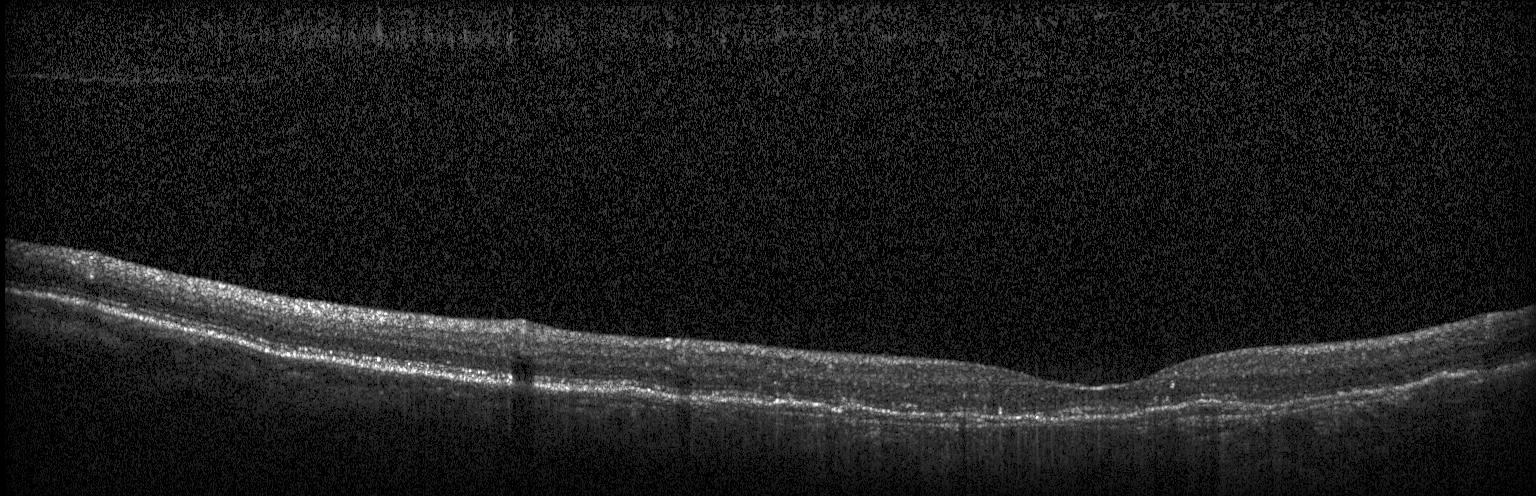 Acquired on a Heidelberg Spectralis; horizontal scan through the fovea; OCT line scan; spectral-domain optical coherence tomography.
The scan shows a choroidal neovascular membrane.